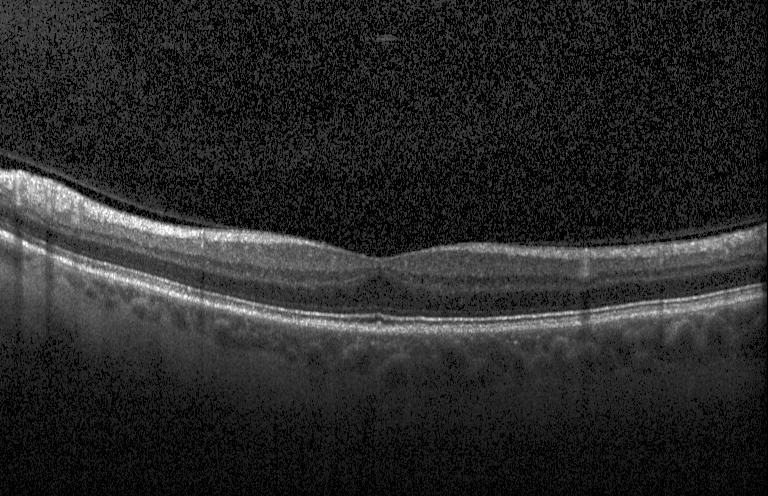
Spectral-domain OCT; OCT line scan — OCT finding: no choroidal neovascularization, no diabetic macular edema, and no drusen.